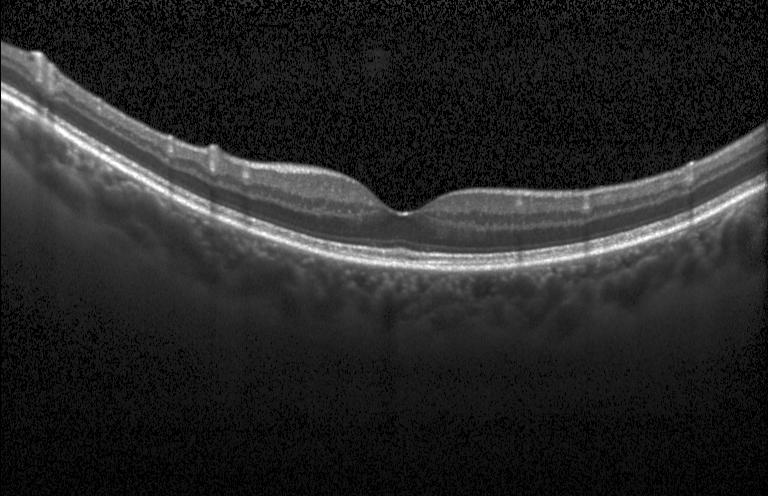 Retinal OCT cross-section — Impression: neither CNV, DME, nor drusen.